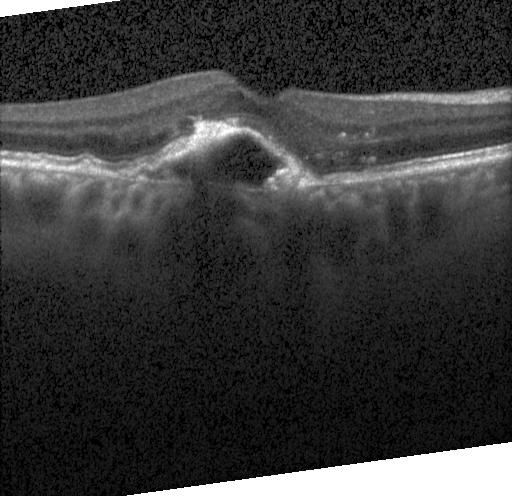 Centered on the fovea · instrument: Heidelberg Spectralis · optical coherence tomography scan.
Impression: choroidal neovascularization (CNV).